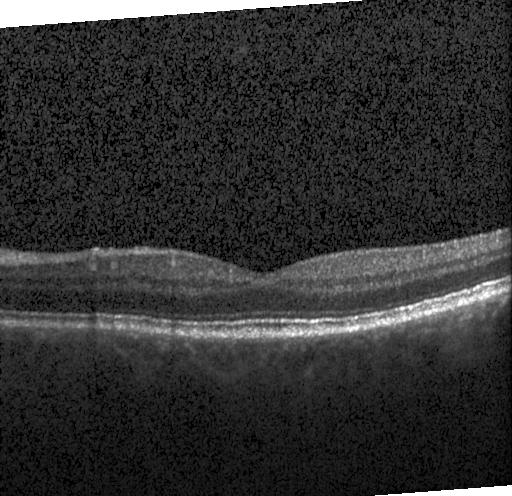
Spectral-domain OCT B-scan: no choroidal neovascularization, no diabetic macular edema, and no drusen.